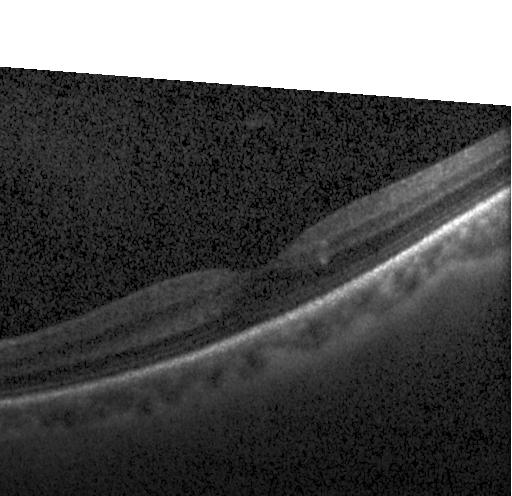

Spectral-domain OCT B-scan: no evidence of CNV, DME, or drusen.